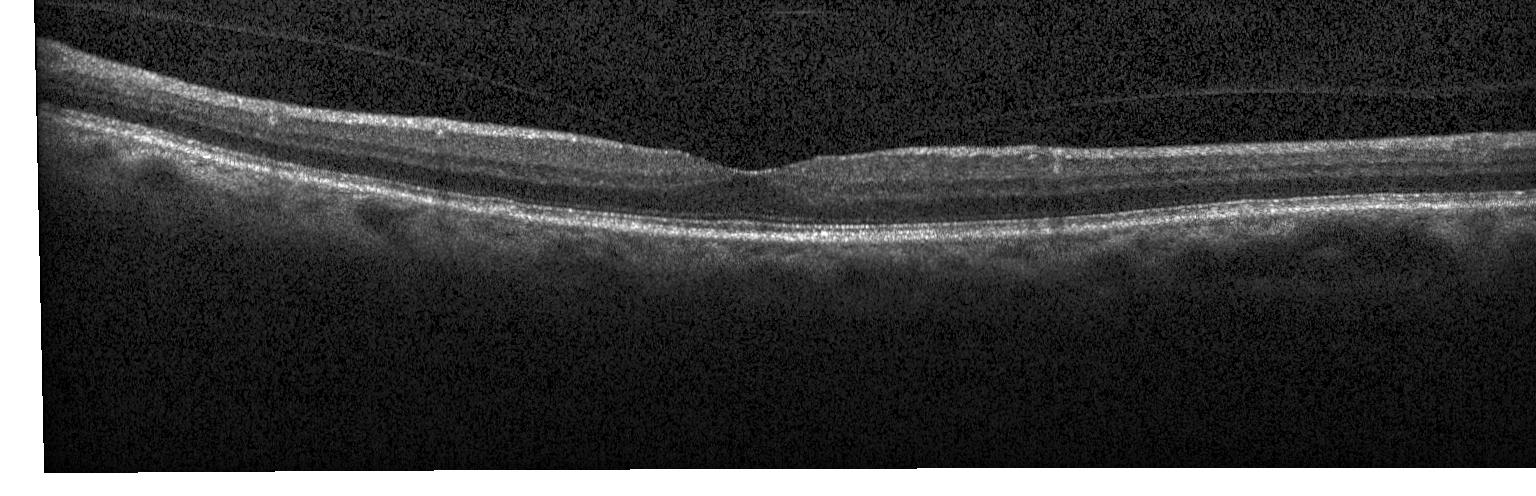 OCT B-scan. Horizontal scan through the fovea. Spectral-domain optical coherence tomography. Heidelberg Spectralis — Finding: no evidence of CNV, DME, or drusen.